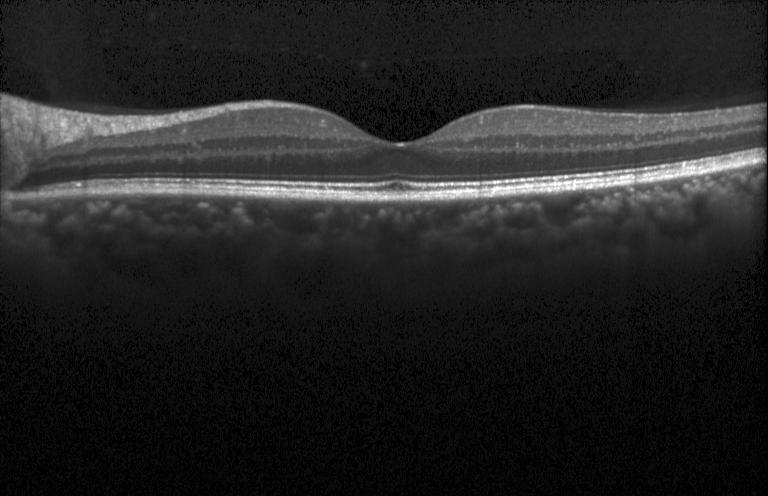 Instrument: Heidelberg Spectralis. Optical coherence tomography scan.
No evidence of choroidal neovascularization, diabetic macular edema, or drusen.